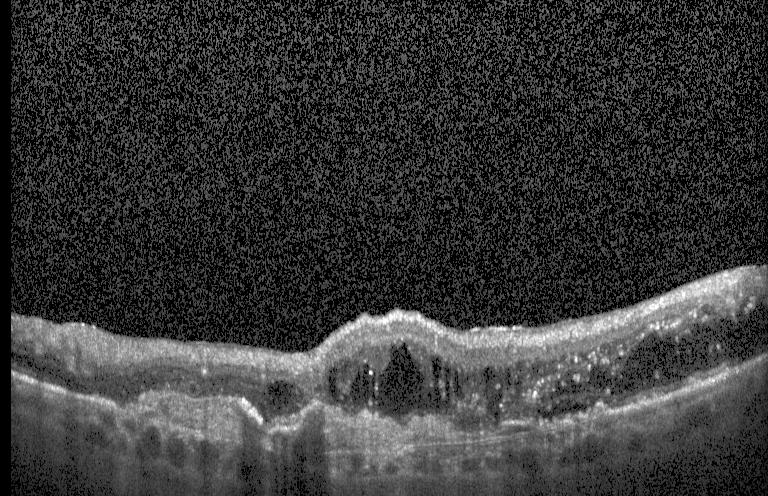 The scan shows a choroidal neovascular membrane.